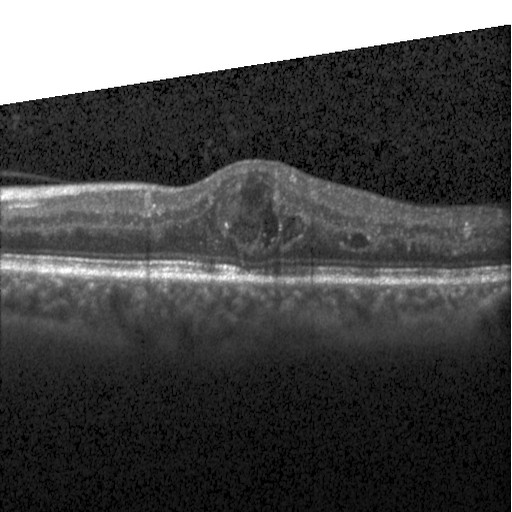
Finding: DME.